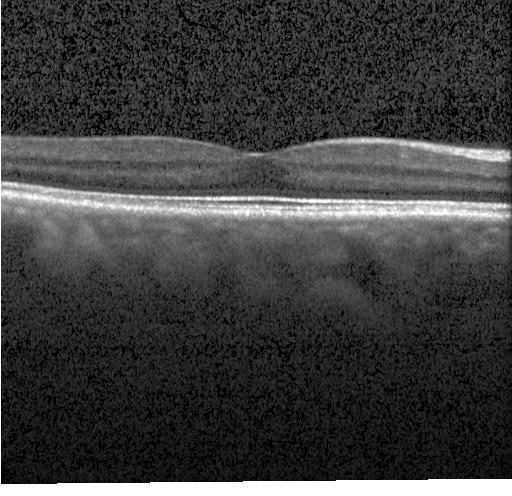
Impression: no evidence of choroidal neovascularization, diabetic macular edema, or drusen.